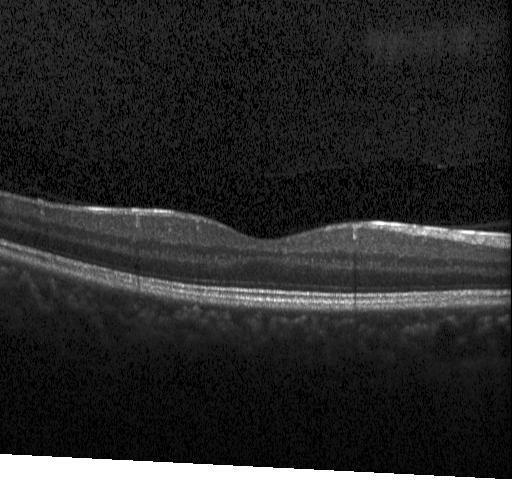

Heidelberg Spectralis OCT system. Retinal OCT B-scan. Spectral-domain optical coherence tomography. Macular scan — Dx: no choroidal neovascularization, diabetic macular edema, or drusen.